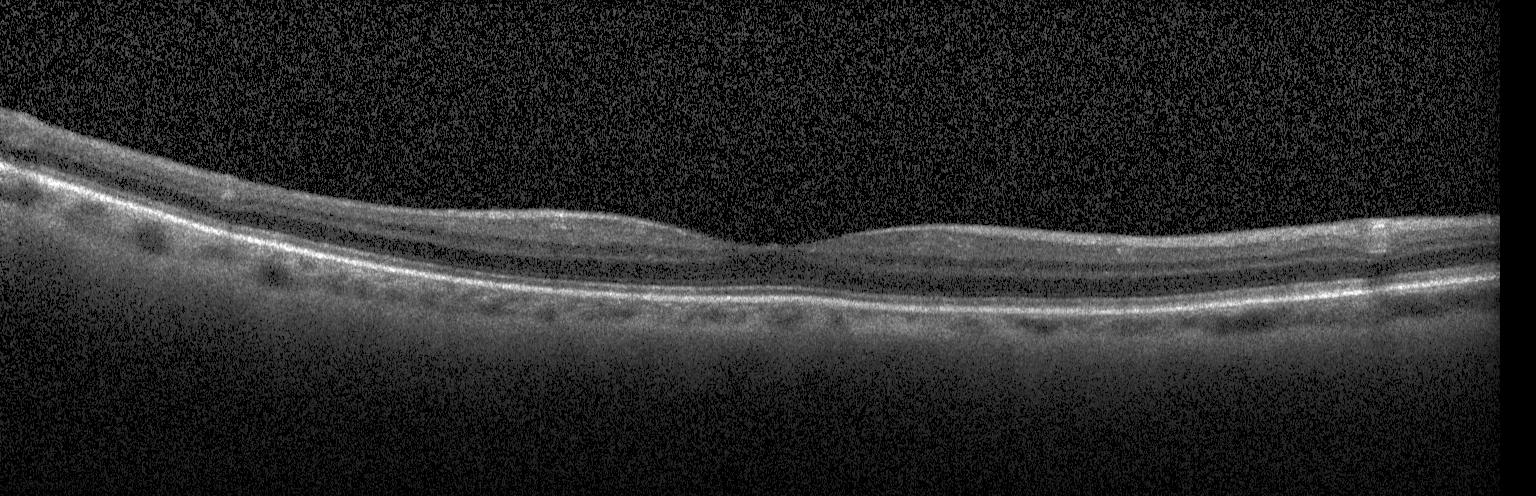 Assessment: no choroidal neovascularization, no diabetic macular edema, and no drusen.